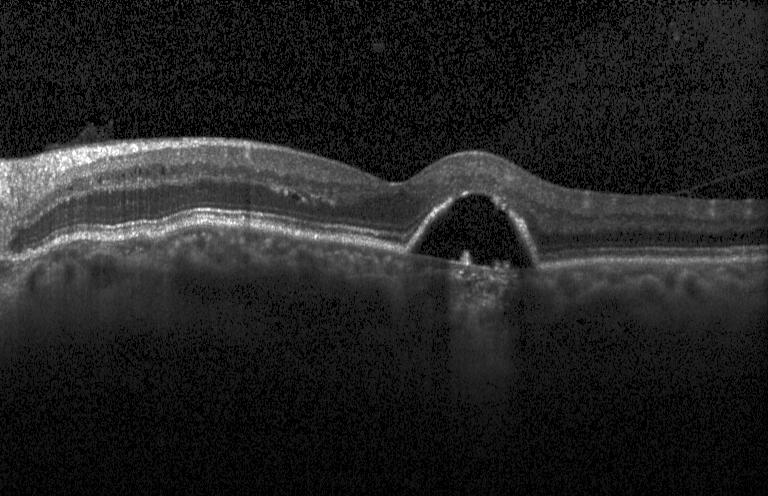

OCT B-scan — OCT finding: CNV.